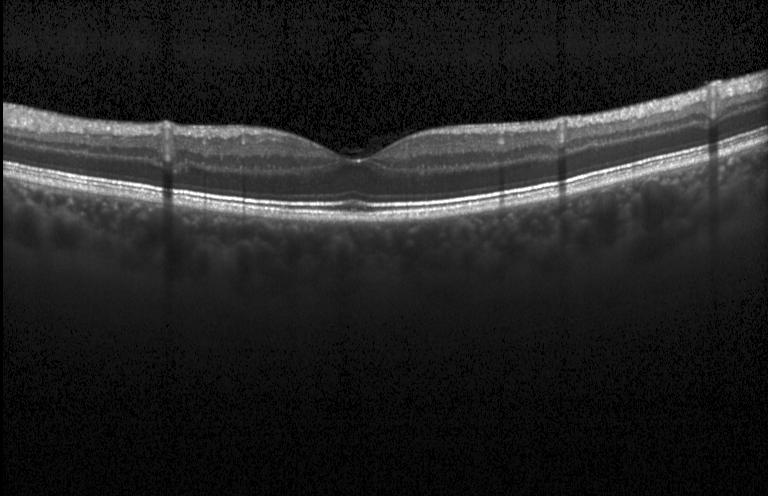

Macular scan. Instrument: Heidelberg Spectralis. Retinal OCT cross-section. Spectral-domain OCT — OCT finding: no evidence of choroidal neovascularization, diabetic macular edema, or drusen.